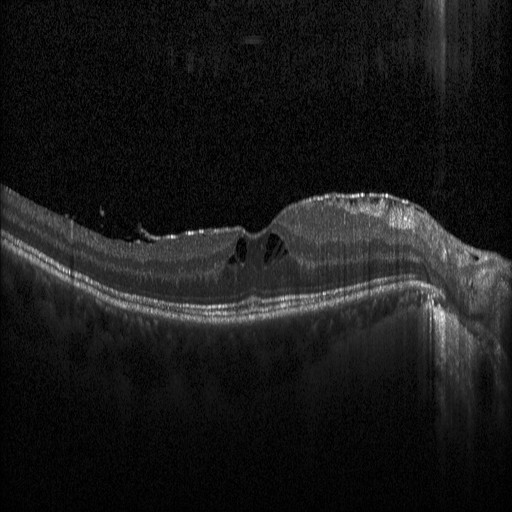

Impression: DME.